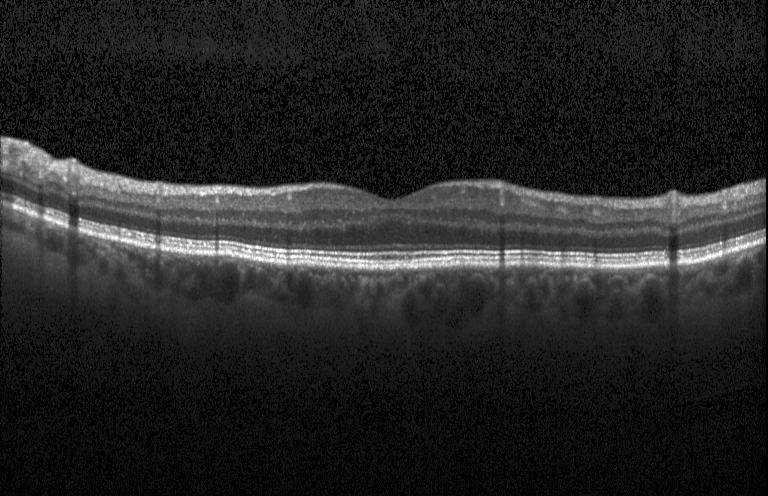 Finding: no CNV, DME, or drusen.